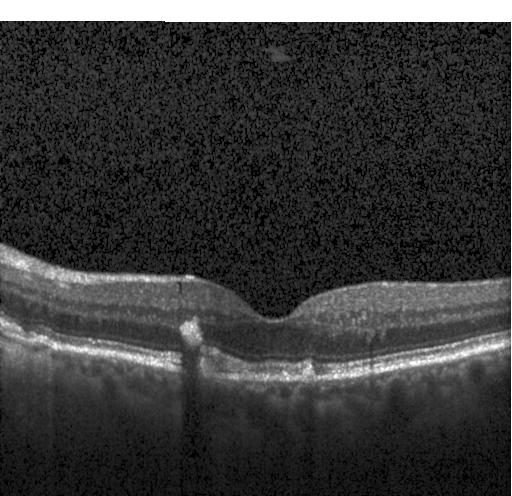
Impression: multiple drusen.